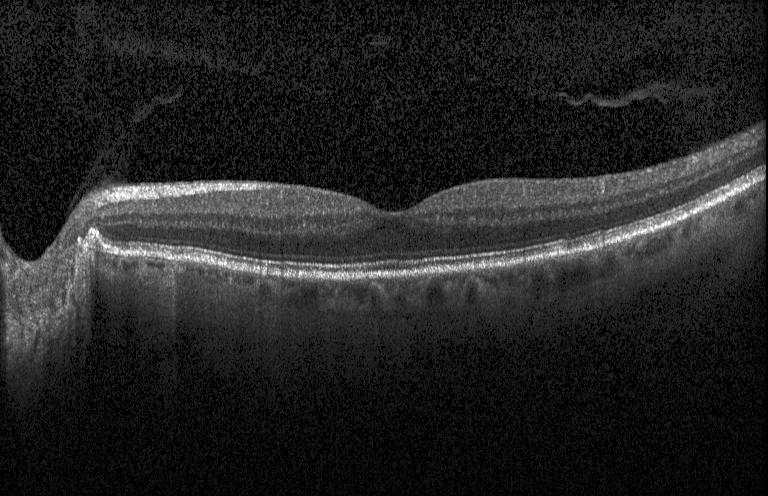
OCT B-scan. SD-OCT
The scan shows no evidence of choroidal neovascularization, diabetic macular edema, or drusen.